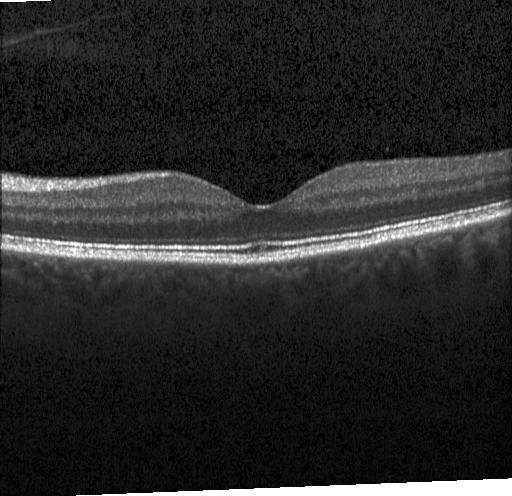
OCT line scan.
Impression: no choroidal neovascularization, no diabetic macular edema, and no drusen.